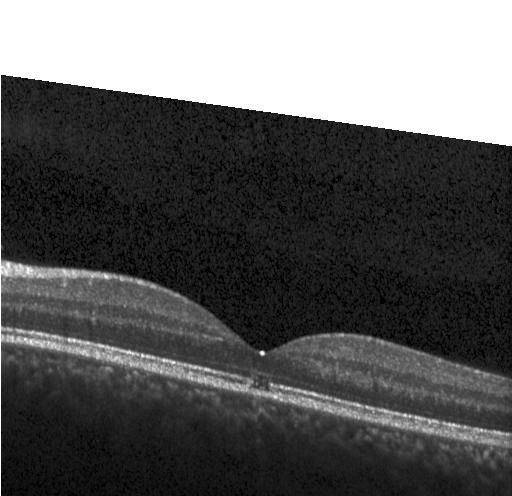

Dx: no CNV, DME, or drusen.